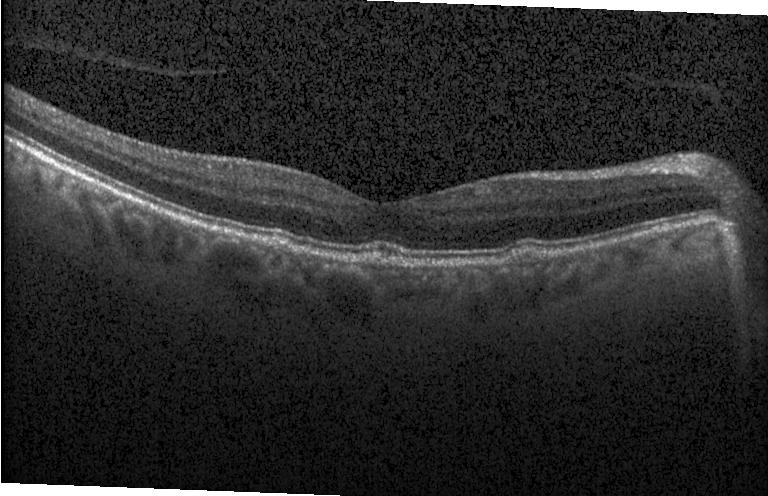

Spectral-domain OCT B-scan: multiple drusen.